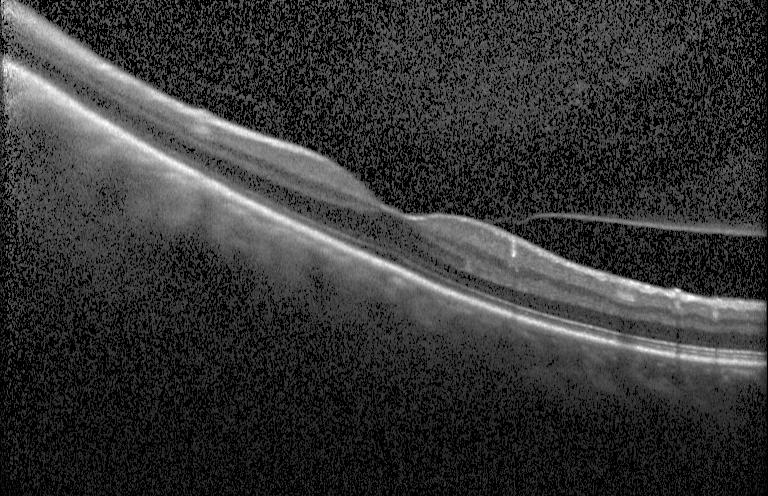
Retinal OCT B-scan
Impression: neither choroidal neovascularization, diabetic macular edema, nor drusen.